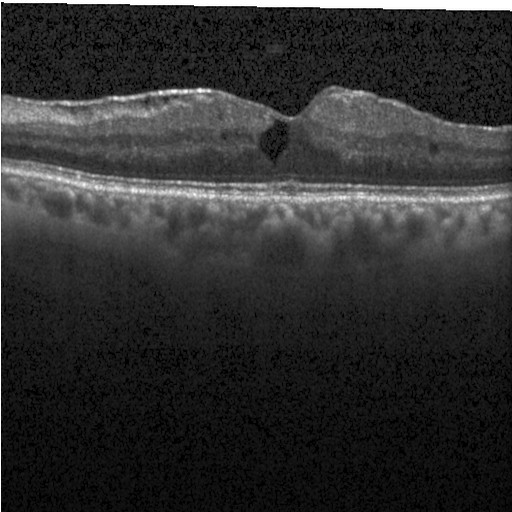
Heidelberg Spectralis; retinal OCT cross-section. OCT finding: diabetic macular edema (DME).